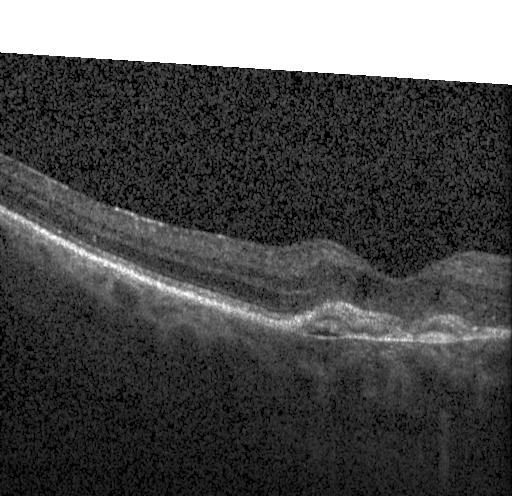
Macular OCT demonstrating a choroidal neovascular membrane.